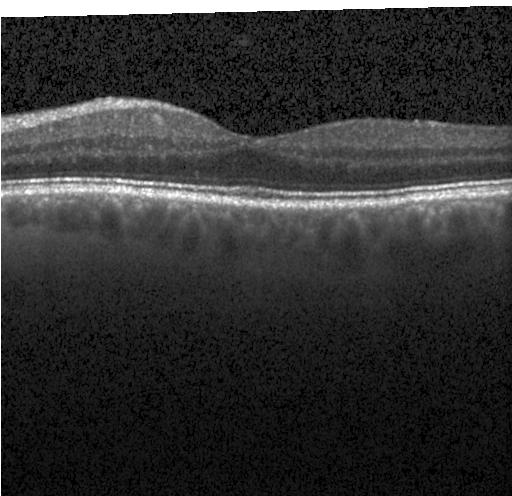 Finding: no choroidal neovascularization, diabetic macular edema, or drusen.